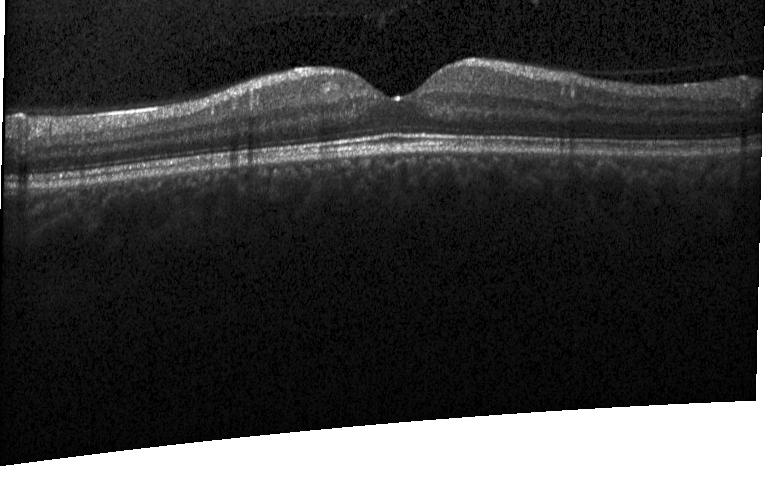 Macular OCT: no evidence of choroidal neovascularization, diabetic macular edema, or drusen.